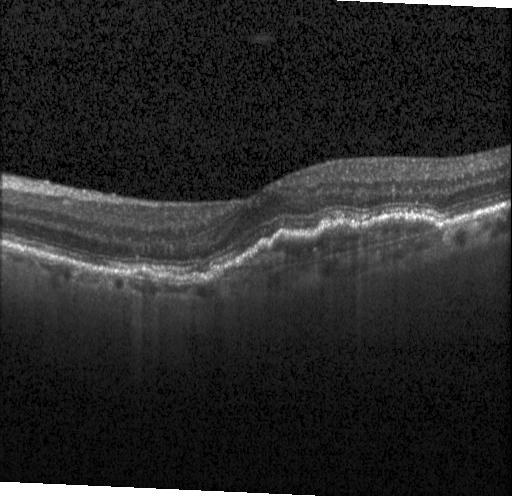 OCT B-scan. Heidelberg Spectralis OCT system. Choroidal neovascularization (CNV).